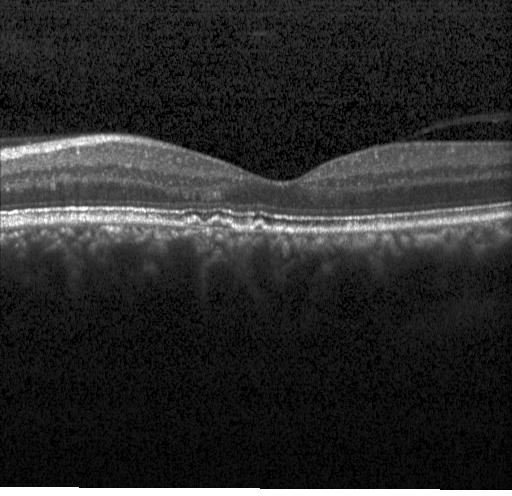
SD-OCT; optical coherence tomography B-scan; instrument: Heidelberg Spectralis.
Dx: drusen.